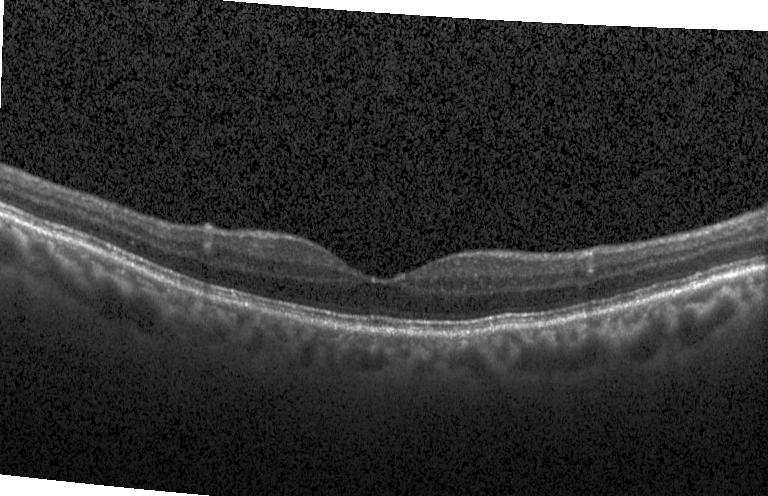
This B-scan demonstrates neither choroidal neovascularization, diabetic macular edema, nor drusen.